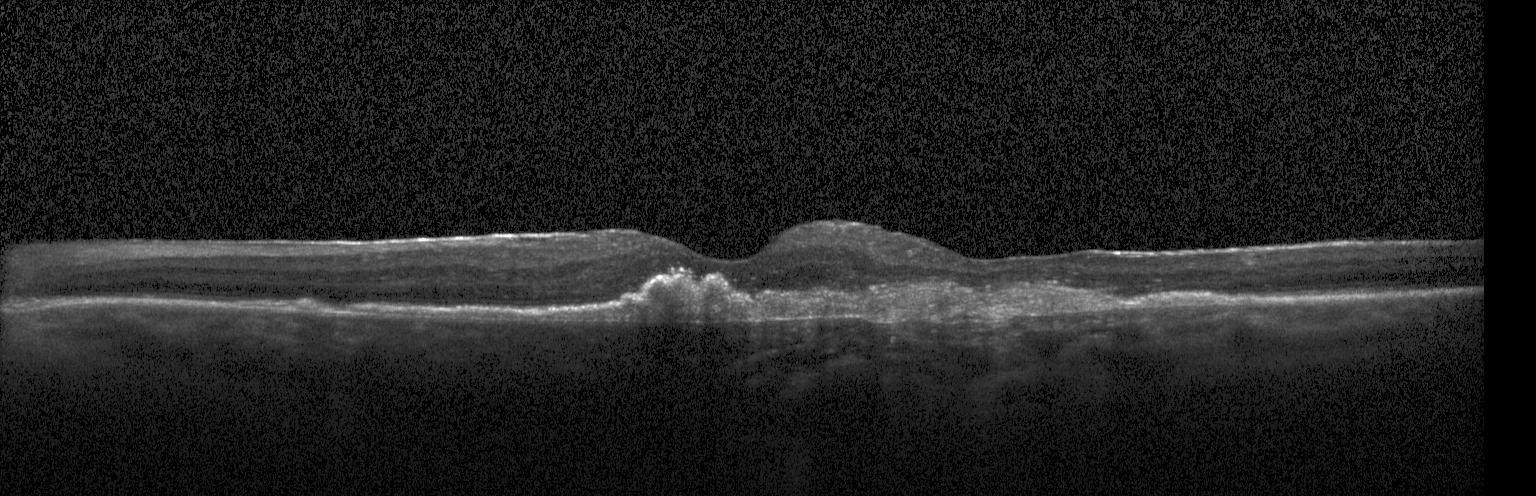

A choroidal neovascular membrane.